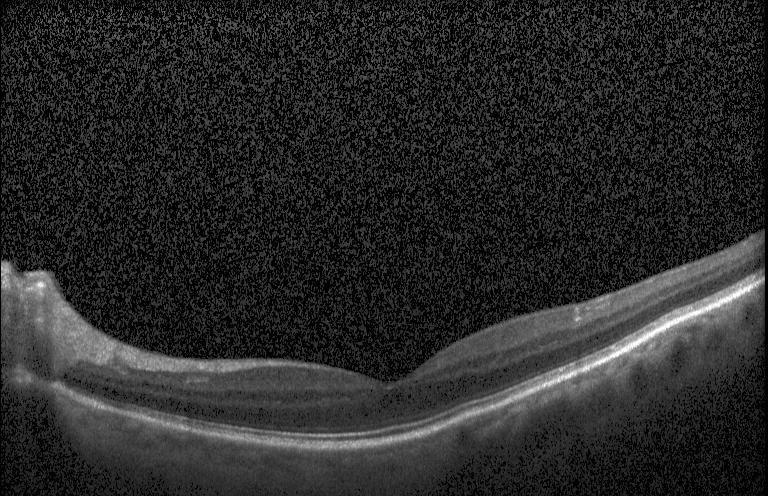 Retinal OCT cross-section. Impression: no choroidal neovascularization, no diabetic macular edema, and no drusen.